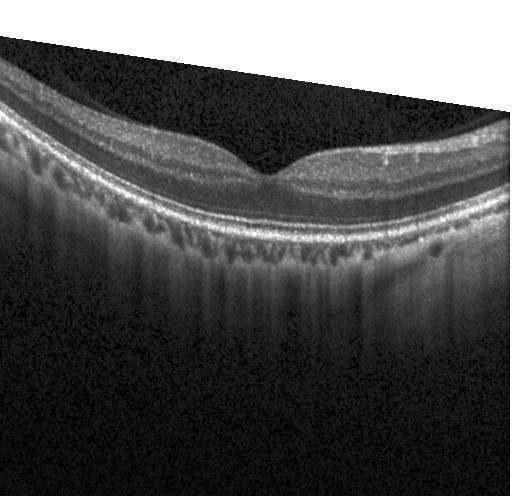

Heidelberg Spectralis · fovea-centered · retinal OCT B-scan
Assessment: no evidence of choroidal neovascularization, diabetic macular edema, or drusen.